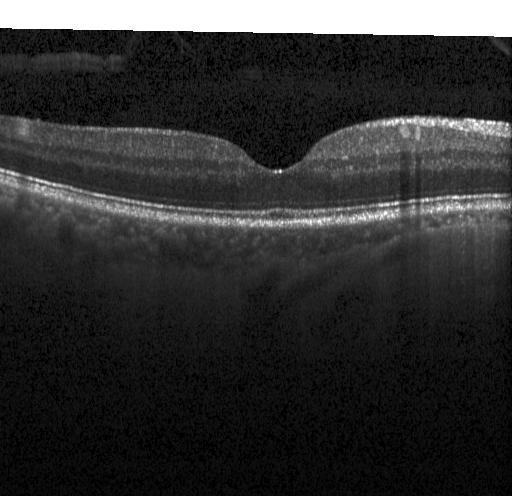 This B-scan demonstrates neither CNV, DME, nor drusen.